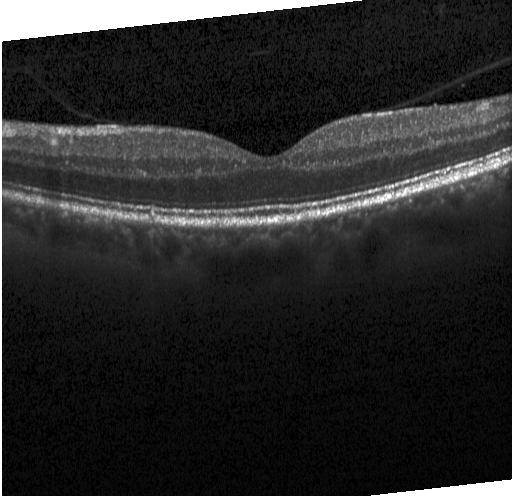
Acquired on a Heidelberg Spectralis, macular scan, spectral-domain optical coherence tomography, retinal OCT B-scan
Diagnosis: no CNV, DME, or drusen.